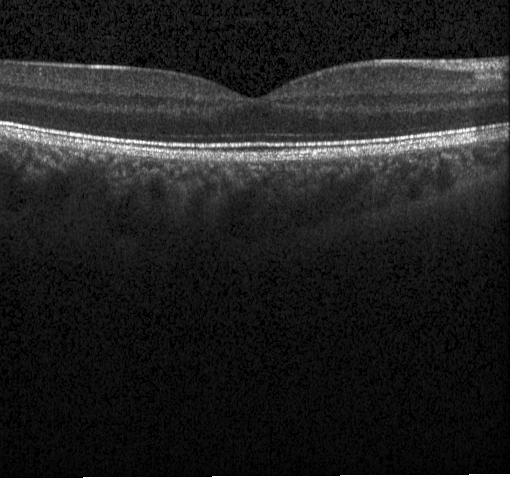
OCT B-scan.
OCT finding: neither choroidal neovascularization, diabetic macular edema, nor drusen.